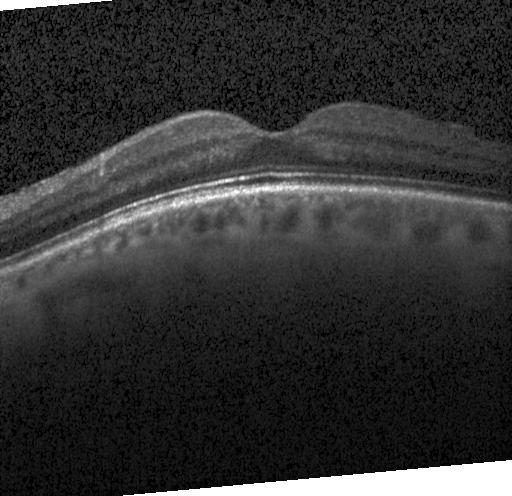
OCT line scan, through the macula, Heidelberg Spectralis, spectral-domain OCT
This B-scan demonstrates no choroidal neovascularization, diabetic macular edema, or drusen.